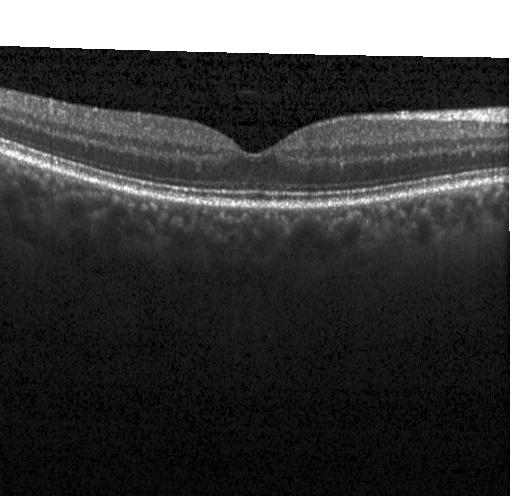 Spectral-domain OCT, retinal OCT B-scan. This B-scan demonstrates neither choroidal neovascularization, diabetic macular edema, nor drusen.